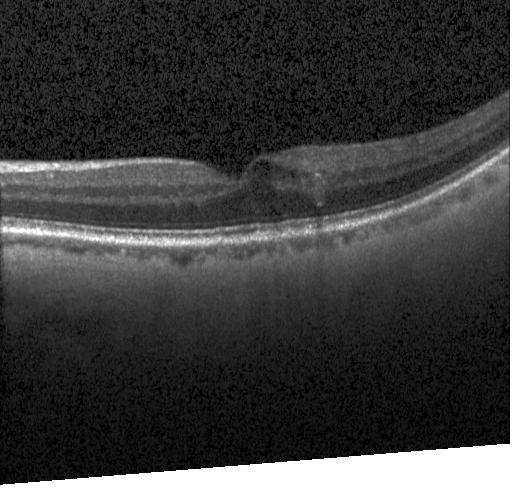

OCT scan showing DME.